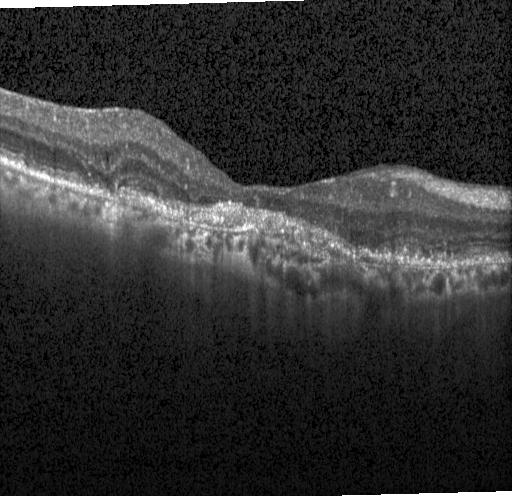

OCT scan showing a choroidal neovascular membrane.